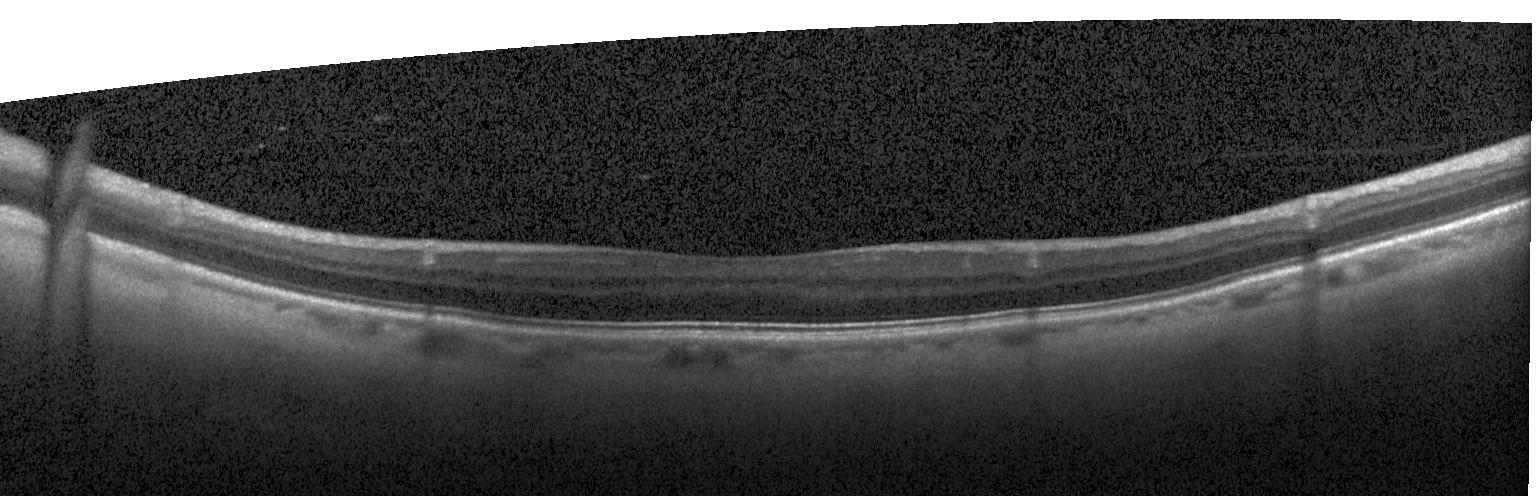

Spectral-domain OCT B-scan: no choroidal neovascularization, diabetic macular edema, or drusen.